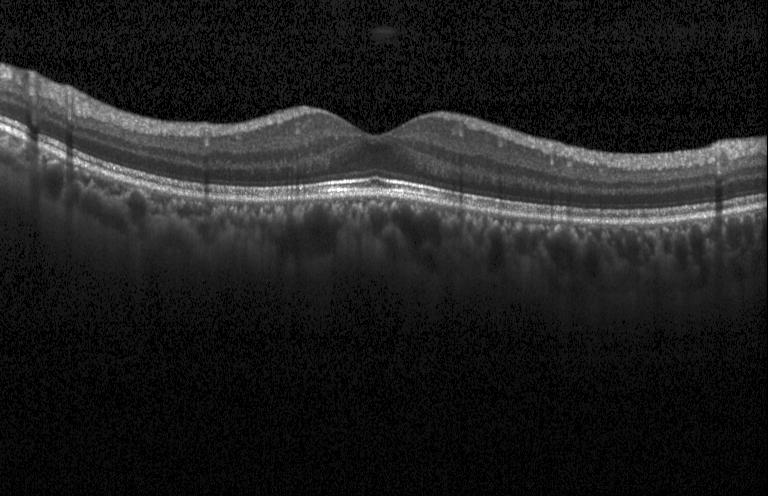 Spectral-domain OCT B-scan: neither choroidal neovascularization, diabetic macular edema, nor drusen.